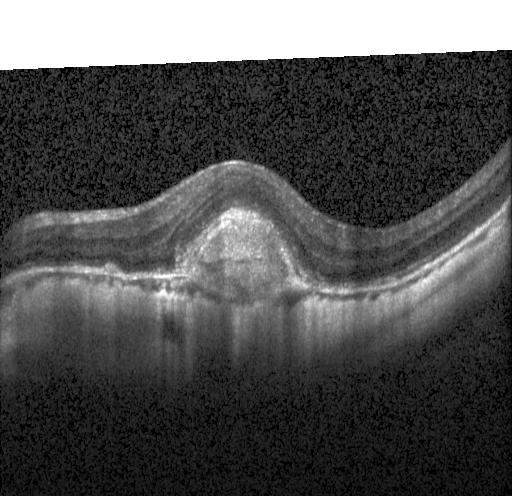
Horizontal scan through the fovea, instrument: Heidelberg Spectralis, SD-OCT, retinal OCT cross-section.
Impression: a choroidal neovascular membrane.